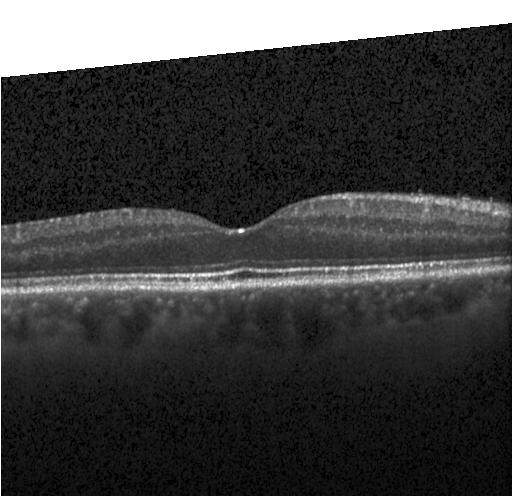 Retinal OCT B-scan, SD-OCT, fovea-centered, instrument: Heidelberg Spectralis — No choroidal neovascularization, diabetic macular edema, or drusen.